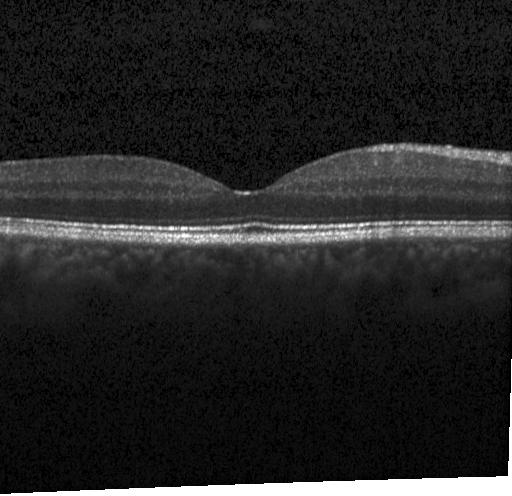 Optical coherence tomography scan. This B-scan demonstrates no choroidal neovascularization, diabetic macular edema, or drusen.